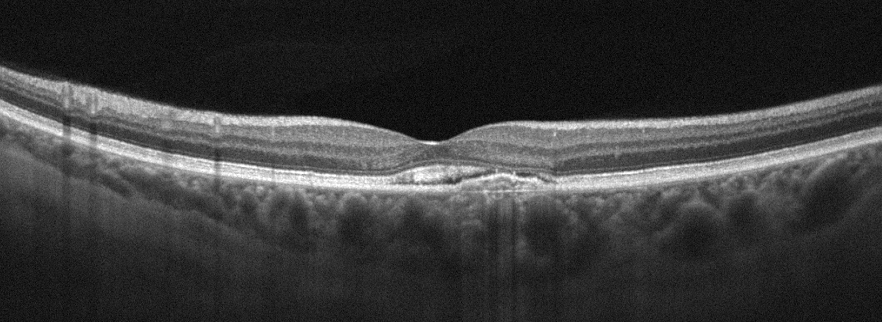

Optical coherence tomography B-scan; left eye — Age-related macular degeneration (AMD).